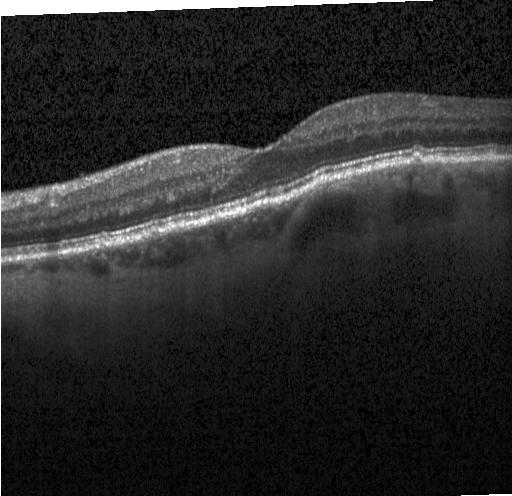
Retinal OCT B-scan
Diagnosis: drusen.